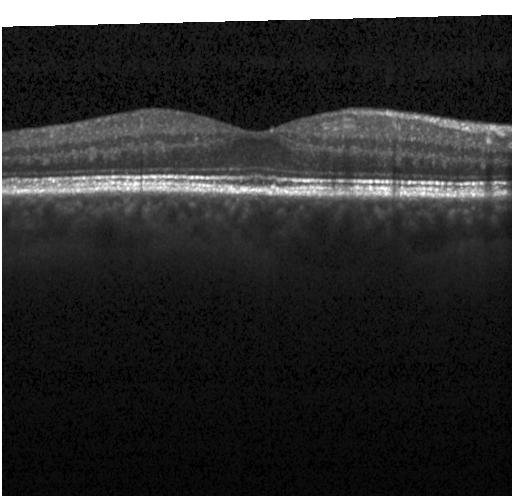

Finding: no choroidal neovascularization, diabetic macular edema, or drusen.